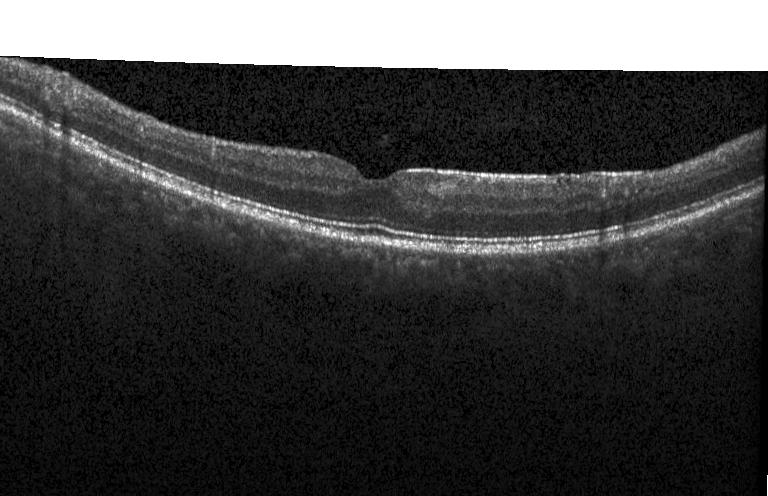
Optical coherence tomography B-scan. Spectral-domain optical coherence tomography. Heidelberg Spectralis
The scan shows no evidence of choroidal neovascularization, diabetic macular edema, or drusen.